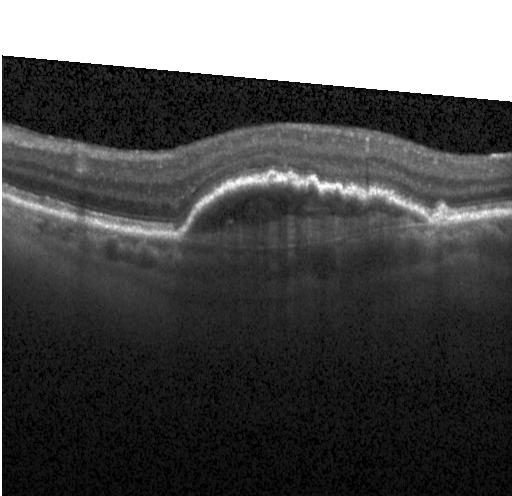 OCT B-scan. Heidelberg Spectralis
Impression: choroidal neovascularization (CNV).